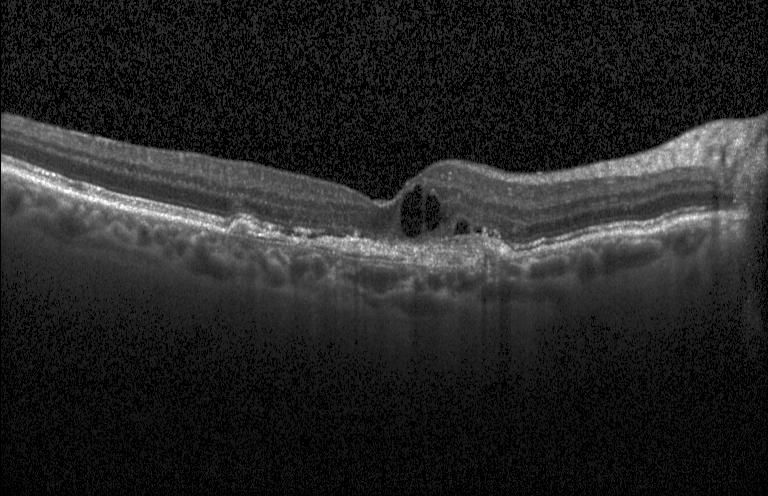 Retinal OCT cross-section. Spectral-domain OCT. Impression: choroidal neovascularization.